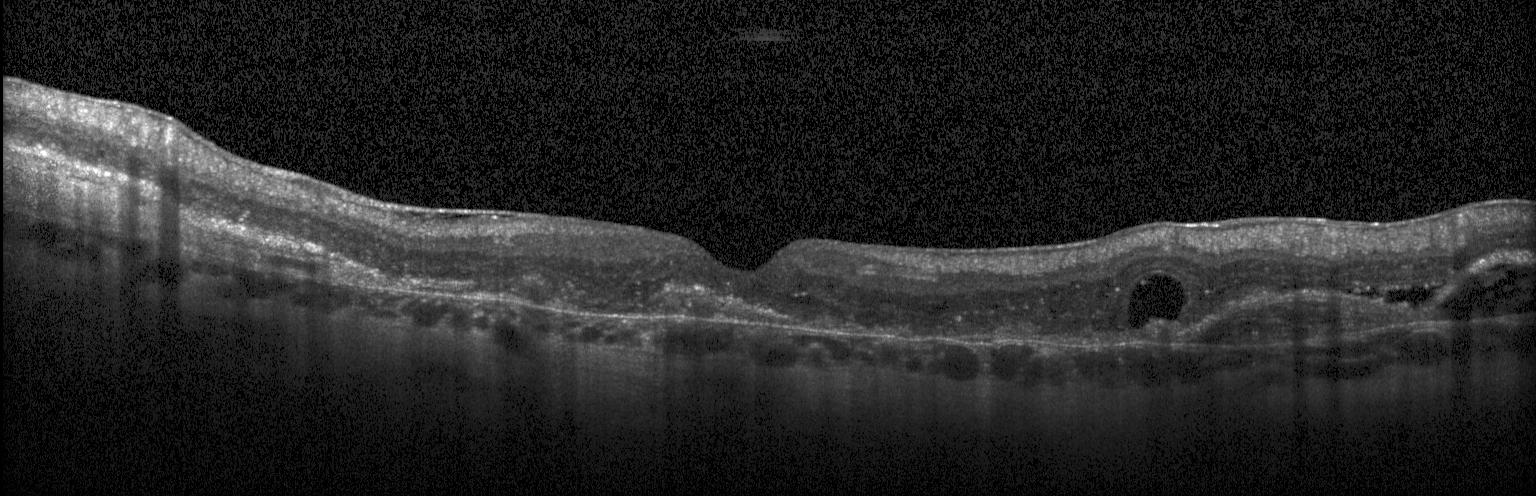 Macular OCT: a choroidal neovascular membrane.